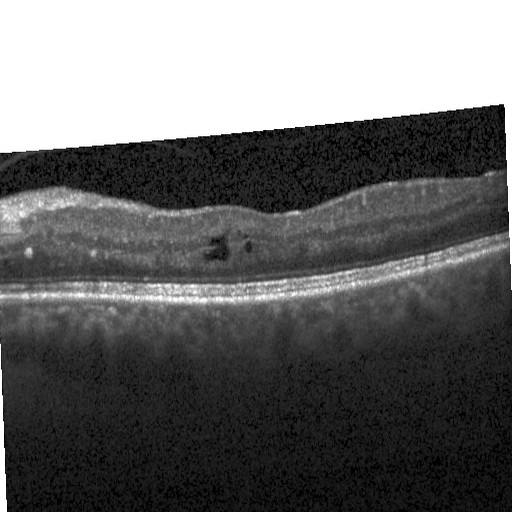

Optical coherence tomography scan, fovea-centered. This B-scan demonstrates DME.